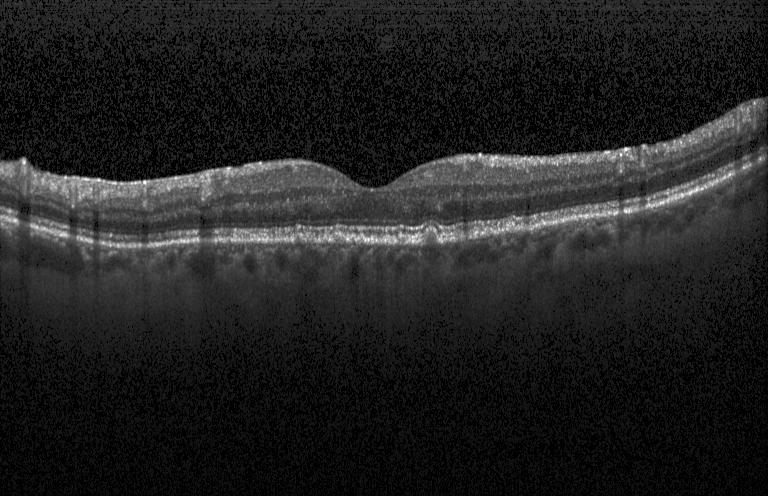 OCT finding: sub-RPE drusenoid deposits.